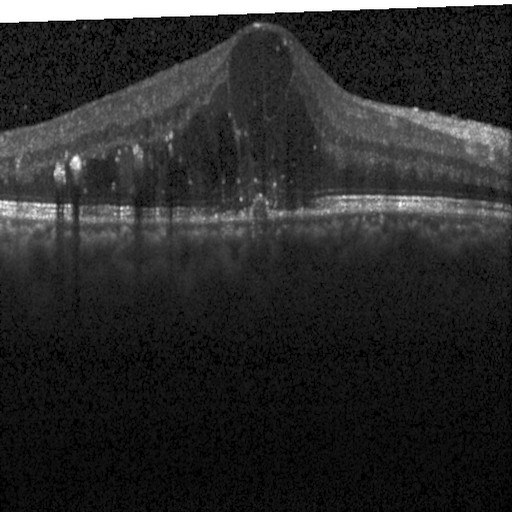

Retinal OCT B-scan — Diagnosis: diabetic macular edema.